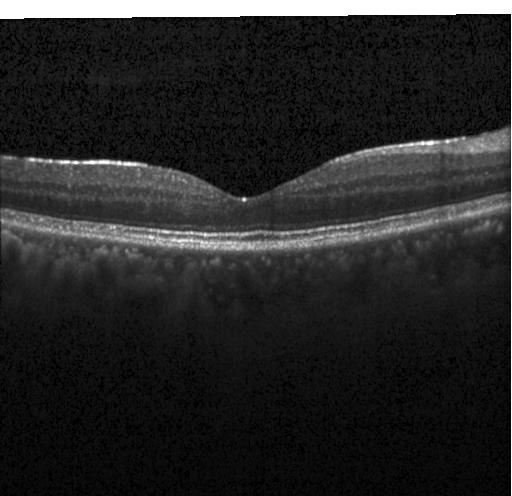
Retinal OCT cross-section; instrument: Heidelberg Spectralis. Impression: no choroidal neovascularization, no diabetic macular edema, and no drusen.